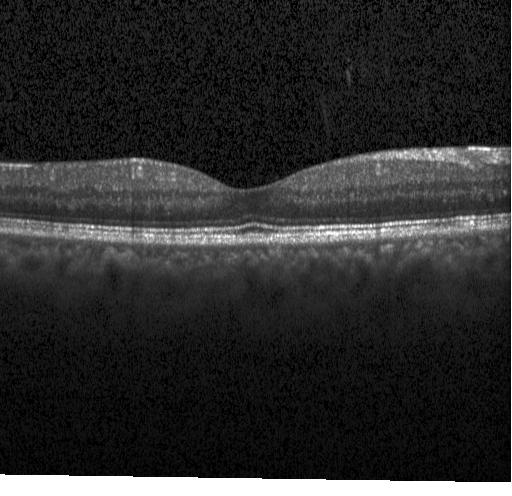
SD-OCT · Heidelberg Spectralis OCT system · retinal OCT cross-section.
Impression: no choroidal neovascularization, no diabetic macular edema, and no drusen.